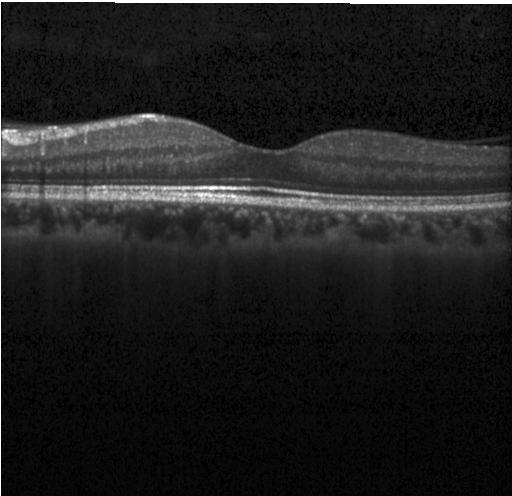 Optical coherence tomography scan — Impression: no CNV, DME, or drusen.